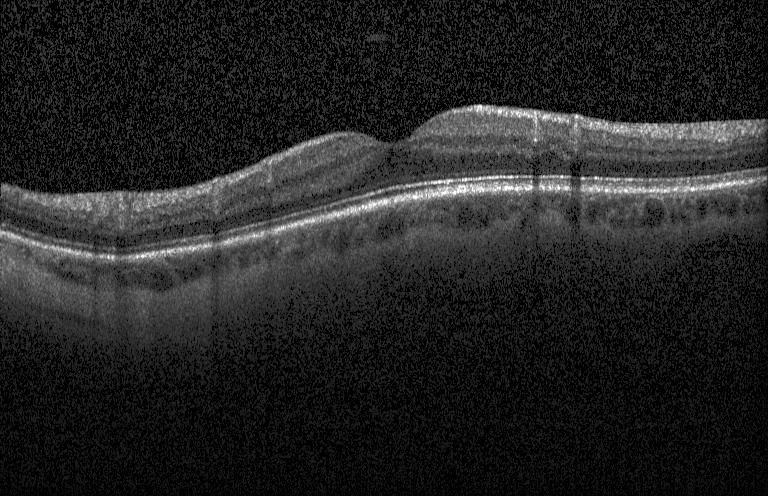
Optical coherence tomography B-scan. SD-OCT. Assessment: no choroidal neovascularization, no diabetic macular edema, and no drusen.